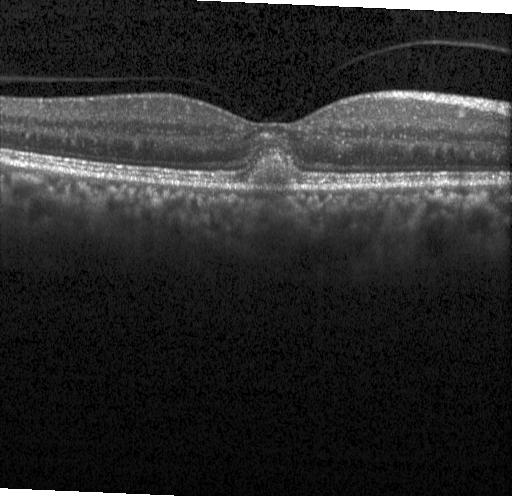
Diagnosis: choroidal neovascularization.